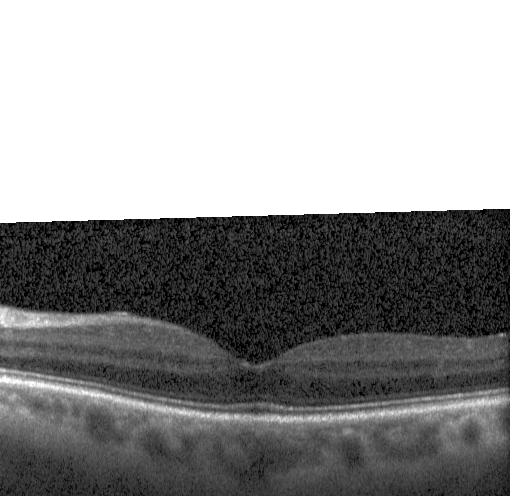 OCT B-scan, acquired on a Heidelberg Spectralis, spectral-domain OCT, fovea-centered
The scan shows neither choroidal neovascularization, diabetic macular edema, nor drusen.